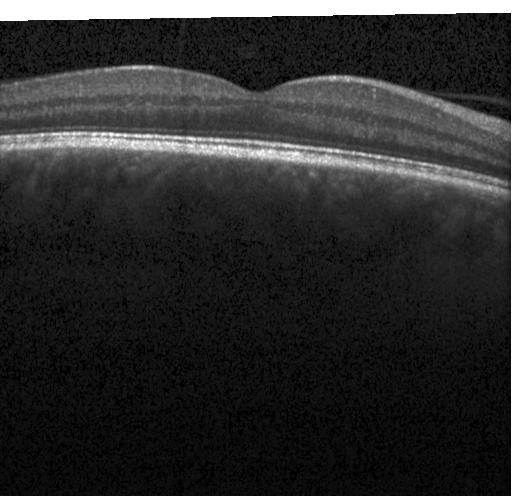

Optical coherence tomography scan — Macular OCT: neither choroidal neovascularization, diabetic macular edema, nor drusen.